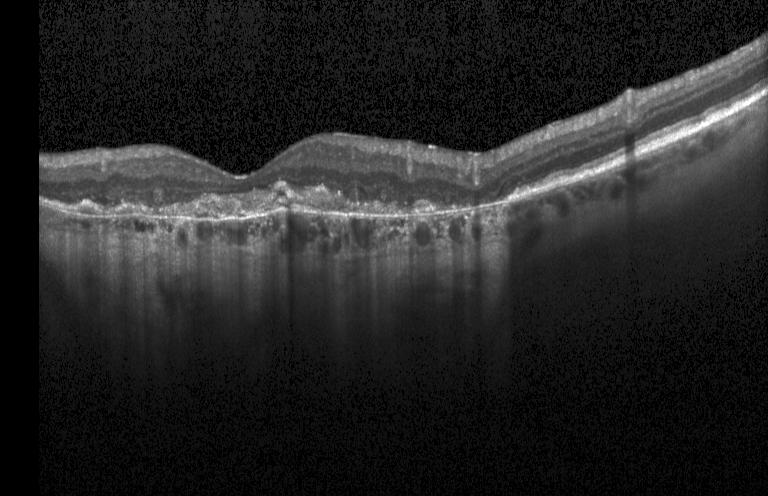 Retinal OCT B-scan · through the macula · Heidelberg Spectralis OCT system — Impression: choroidal neovascularization (CNV).